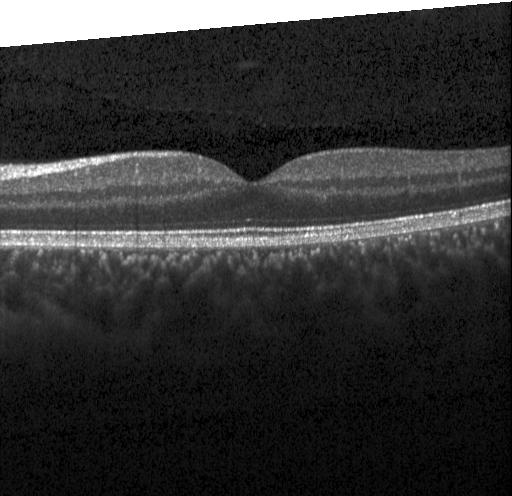
Spectral-domain OCT B-scan: no evidence of choroidal neovascularization, diabetic macular edema, or drusen.